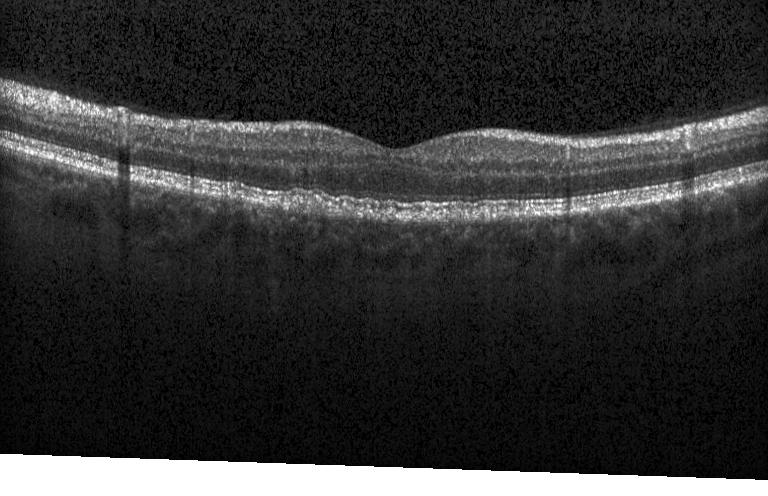

Finding: multiple drusen.